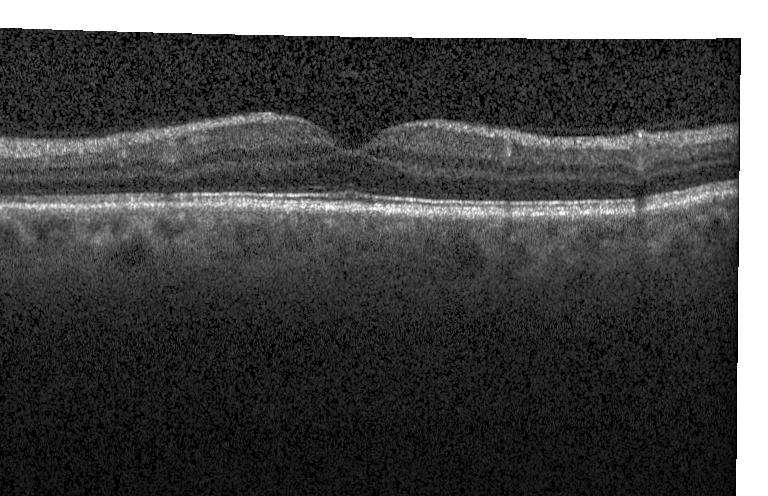 Retinal OCT cross-section, through the macula
Finding: no evidence of choroidal neovascularization, diabetic macular edema, or drusen.